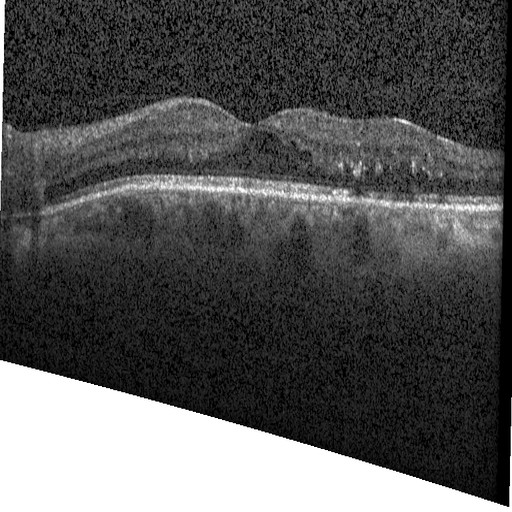 OCT B-scan — Assessment: diabetic macular edema (DME).